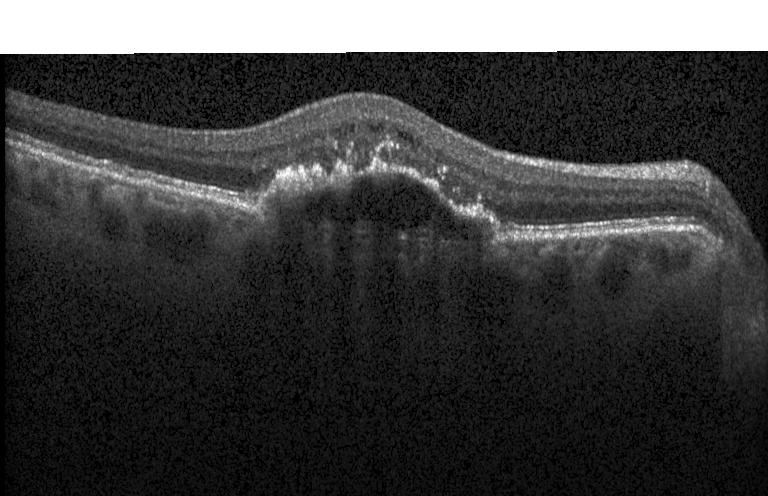
Diagnosis: choroidal neovascularization.